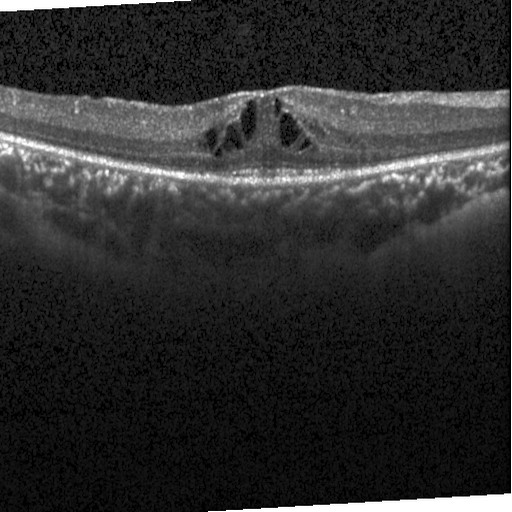 Impression: DME.